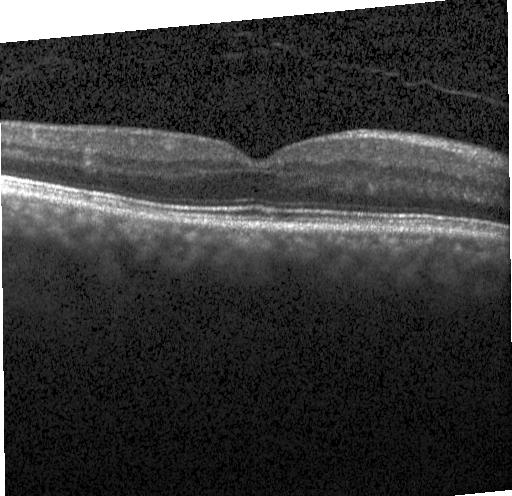
Spectral-domain OCT, optical coherence tomography scan. Impression: no choroidal neovascularization, no diabetic macular edema, and no drusen.